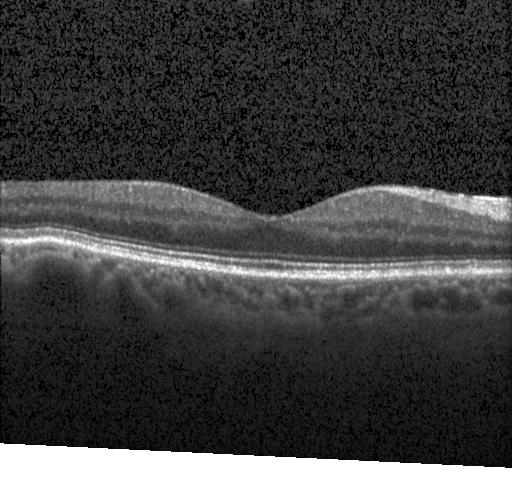

Heidelberg Spectralis; OCT line scan; fovea-centered
This B-scan demonstrates neither choroidal neovascularization, diabetic macular edema, nor drusen.